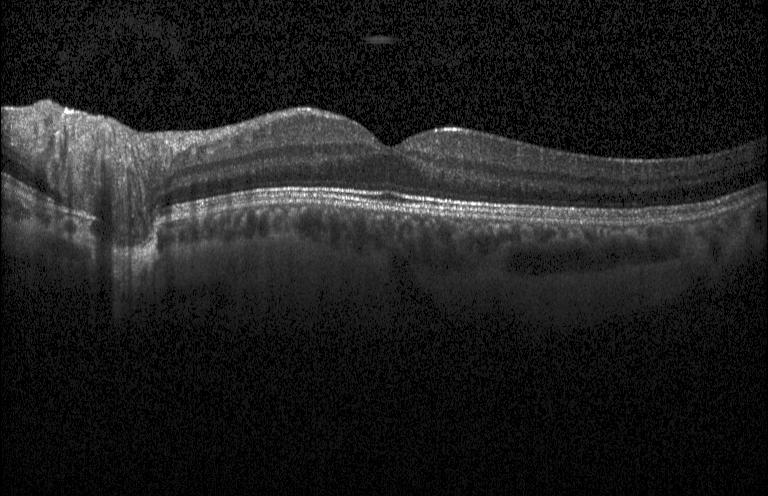
Acquired on a Heidelberg Spectralis, spectral-domain optical coherence tomography, through the macula, retinal OCT cross-section — Macular OCT: no evidence of choroidal neovascularization, diabetic macular edema, or drusen.